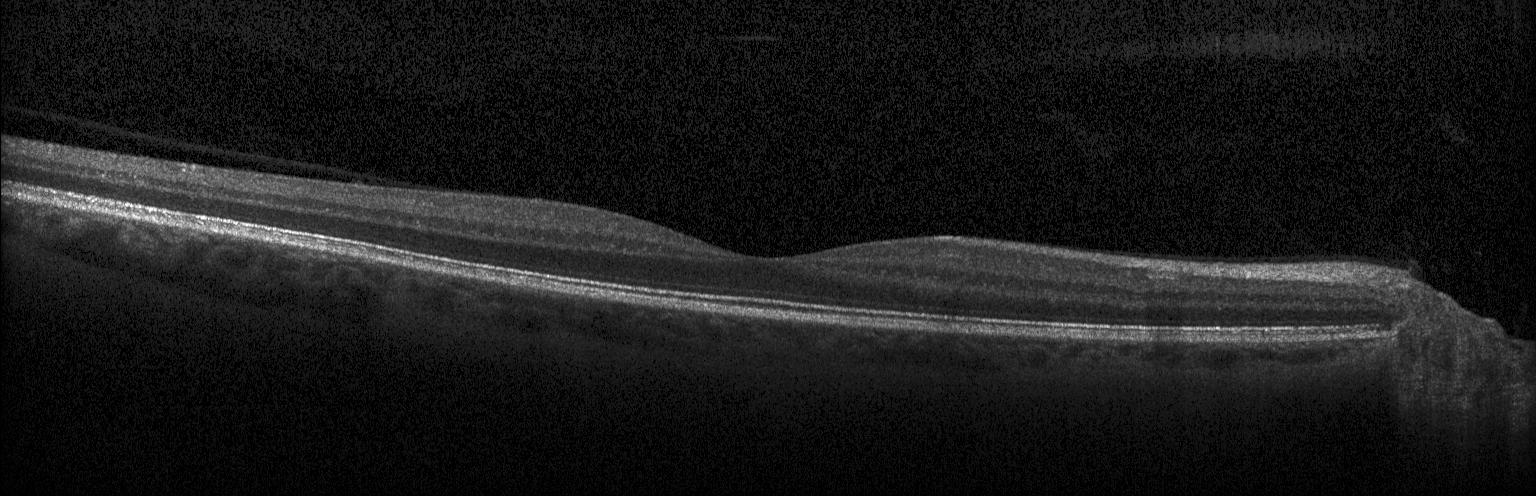

OCT B-scan. Heidelberg Spectralis OCT system. Spectral-domain optical coherence tomography.
Diagnosis: no choroidal neovascularization, no diabetic macular edema, and no drusen.